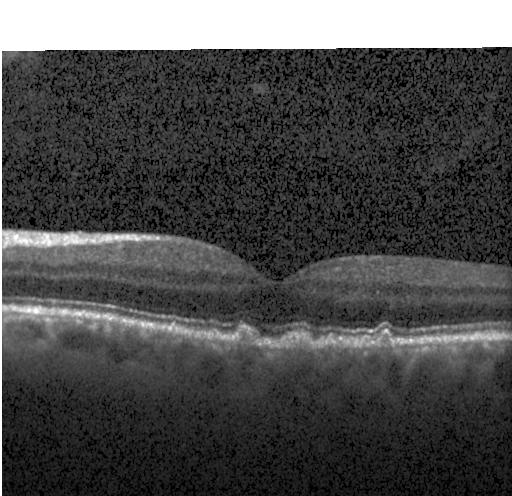 Dx: multiple drusen.